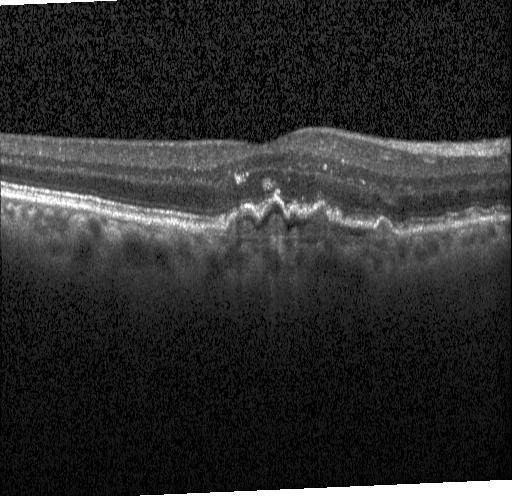 Spectral-domain optical coherence tomography. OCT B-scan — Impression: choroidal neovascularization (CNV).